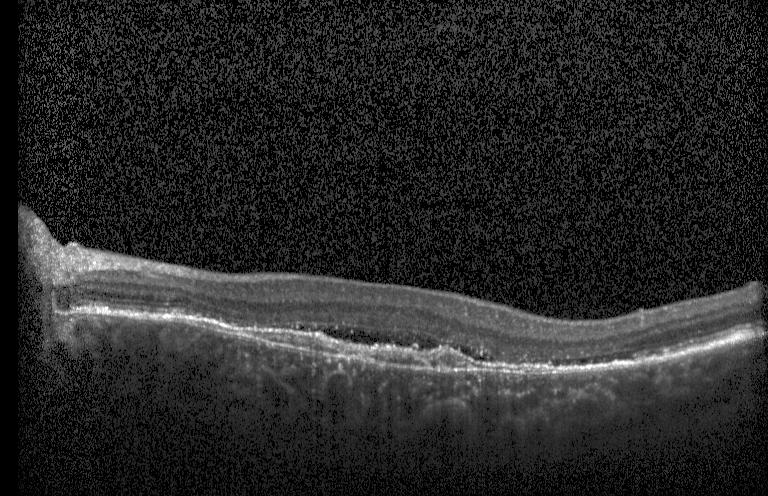
Instrument: Heidelberg Spectralis · spectral-domain optical coherence tomography · retinal OCT B-scan · macular scan — Diagnosis: a choroidal neovascular membrane.